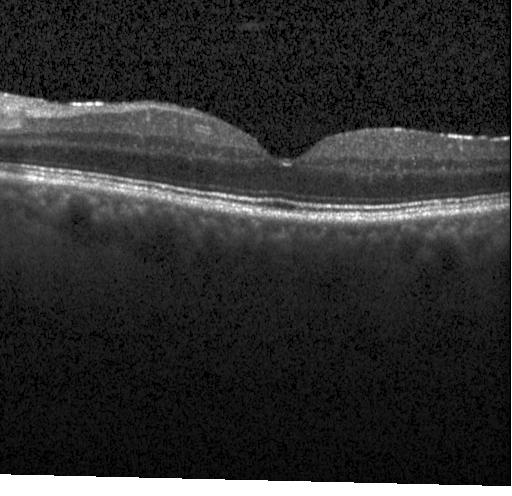 Instrument: Heidelberg Spectralis. Through the macula. Retinal OCT cross-section — Impression: no evidence of CNV, DME, or drusen.